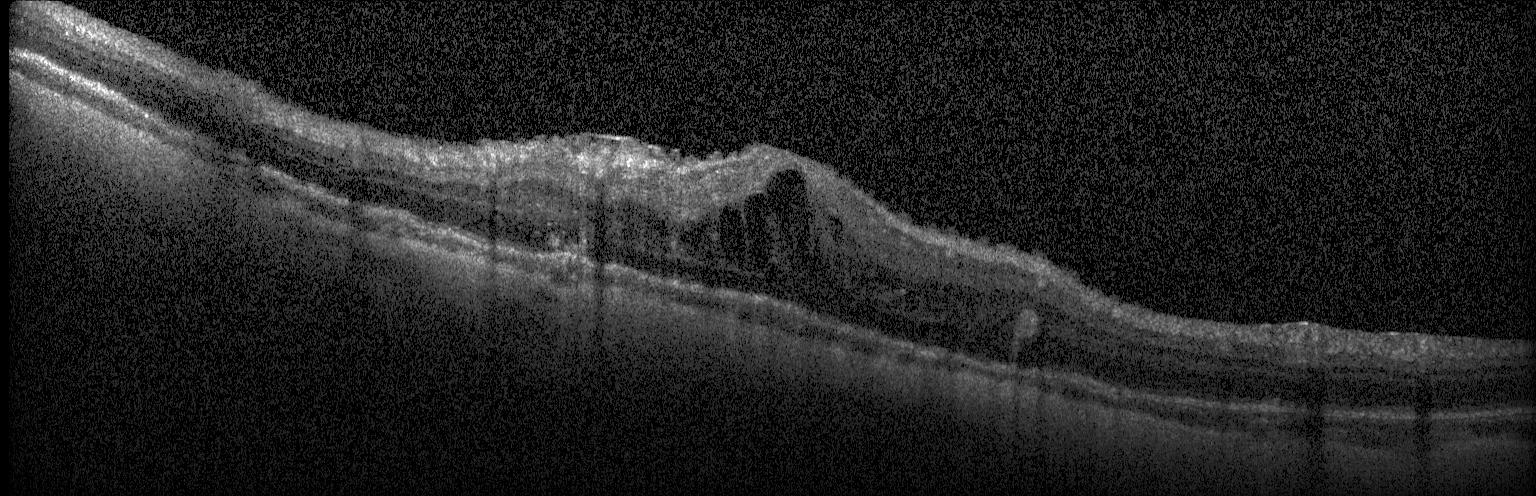
OCT scan showing diabetic macular edema.